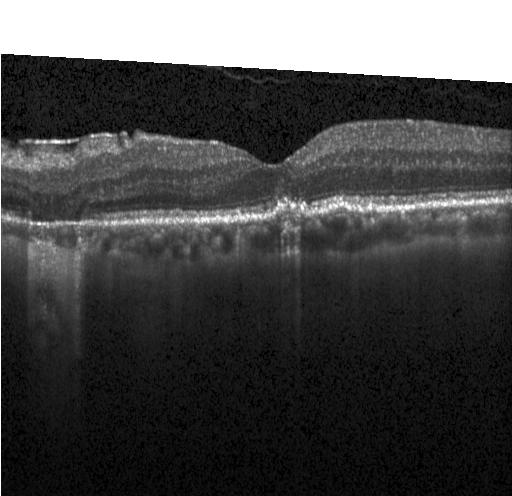

Through the macula; spectral-domain OCT; OCT B-scan — This B-scan demonstrates sub-RPE drusenoid deposits.